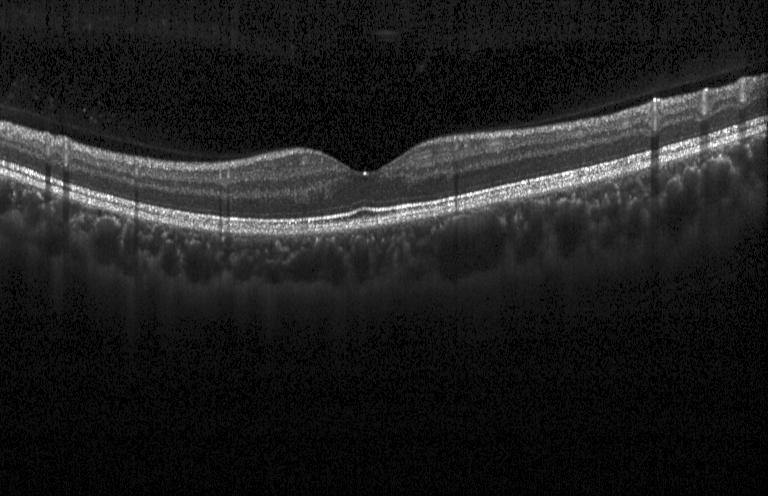

OCT B-scan showing neither choroidal neovascularization, diabetic macular edema, nor drusen.